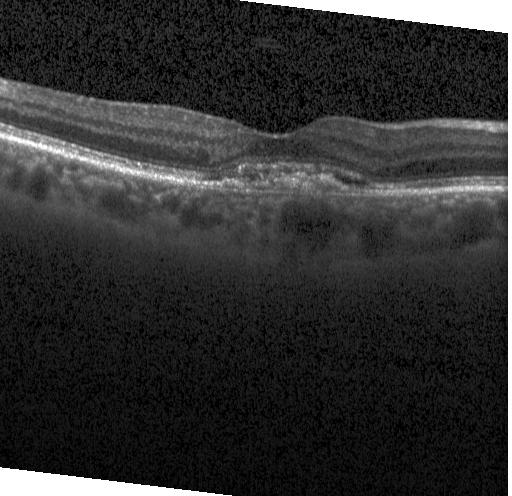

OCT B-scan showing choroidal neovascularization.